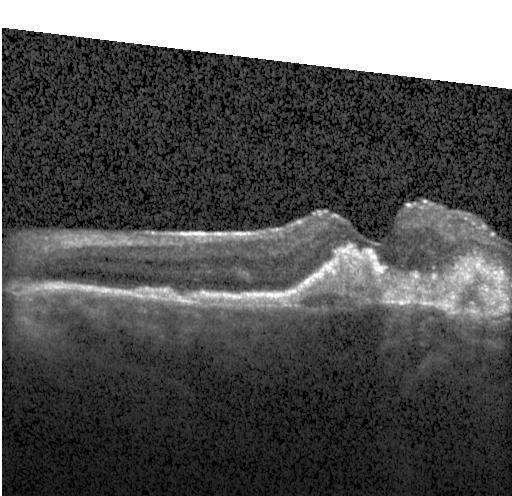 Optical coherence tomography scan, instrument: Heidelberg Spectralis, centered on the fovea. The scan shows a choroidal neovascular membrane.